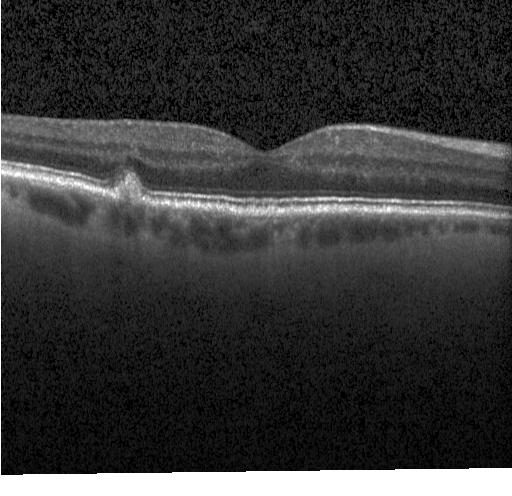

Retinal OCT B-scan · spectral-domain OCT · macular scan
Finding: drusen.